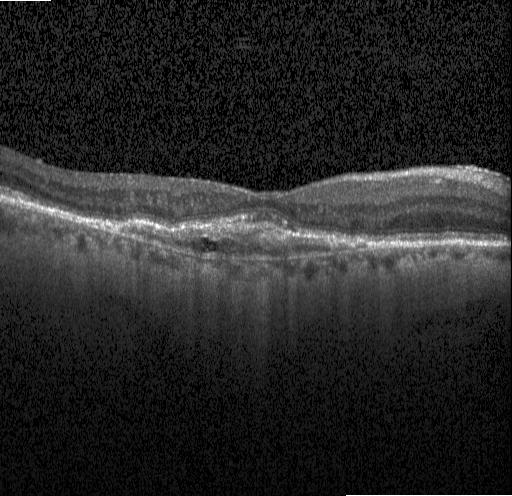
Retinal OCT B-scan; fovea-centered
Finding: a choroidal neovascular membrane.